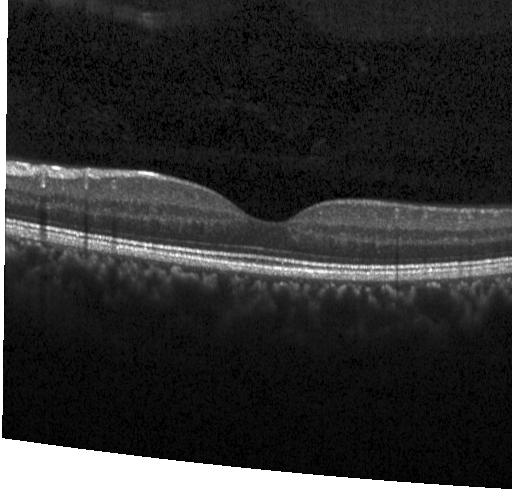 This B-scan demonstrates no CNV, no DME, and no drusen.